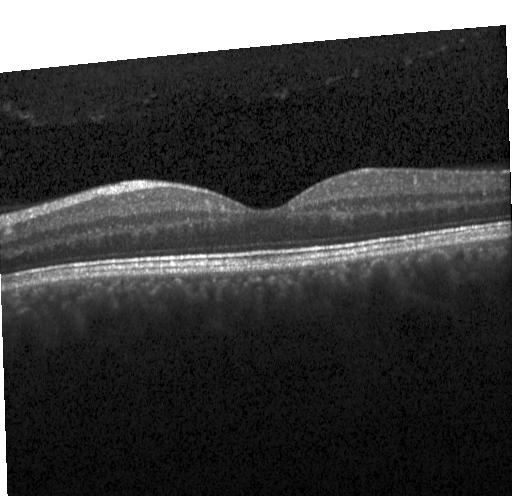
Retinal OCT B-scan. Finding: neither choroidal neovascularization, diabetic macular edema, nor drusen.